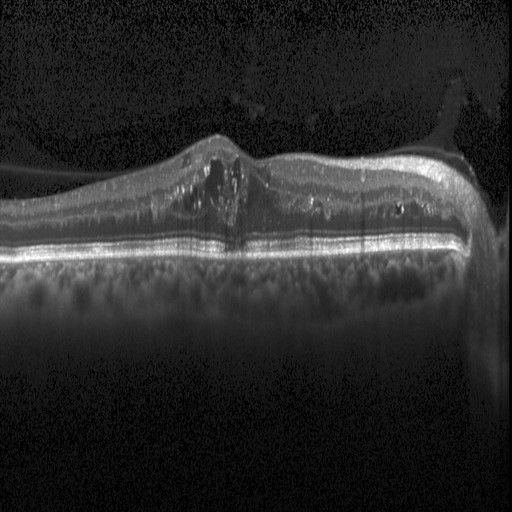

Spectral-domain optical coherence tomography. Optical coherence tomography scan. Through the macula. Instrument: Heidelberg Spectralis — Diagnosis: diabetic macular edema.